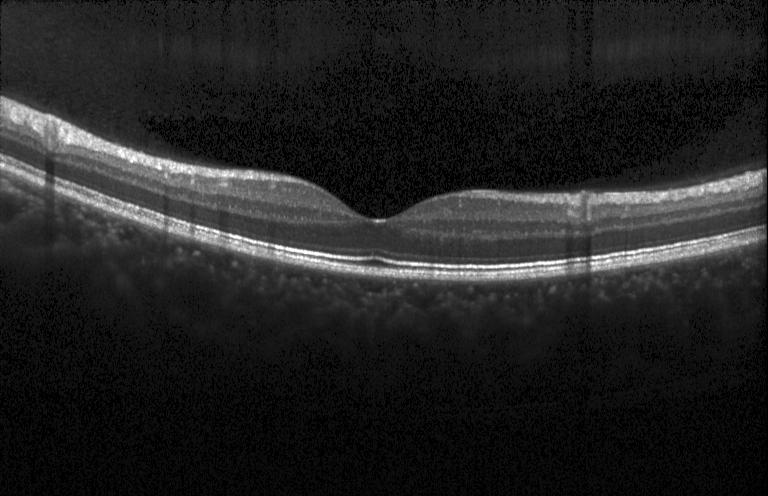

Macular OCT: no choroidal neovascularization, no diabetic macular edema, and no drusen.